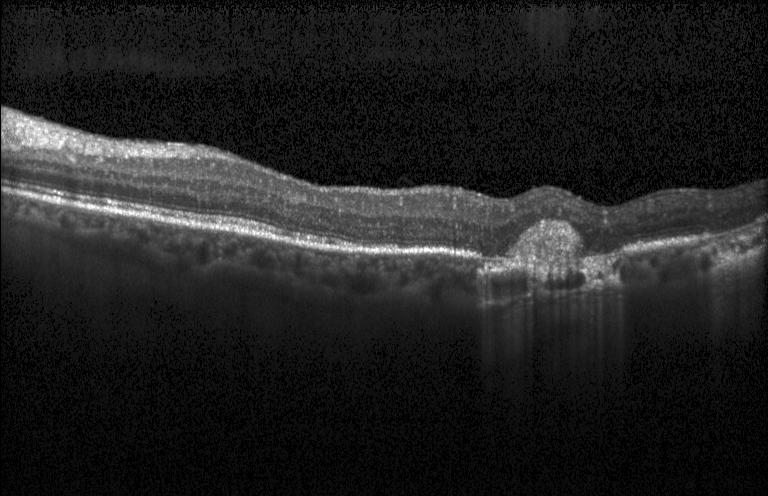
Optical coherence tomography B-scan, Heidelberg Spectralis, centered on the fovea, spectral-domain optical coherence tomography. The scan shows a choroidal neovascular membrane.